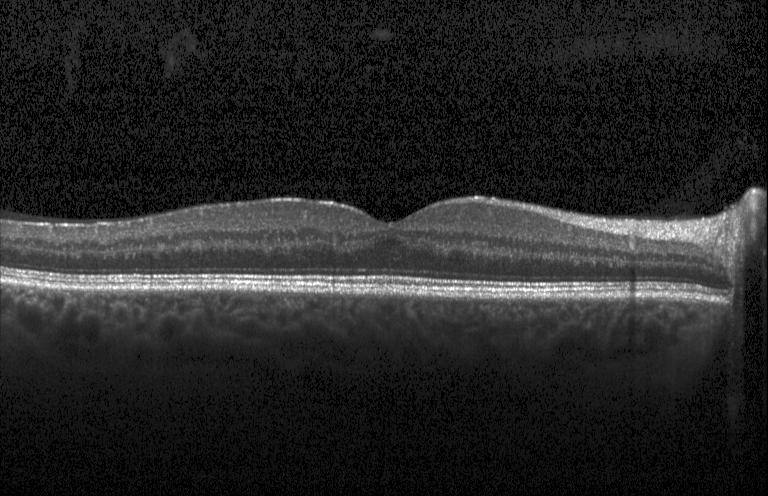 Optical coherence tomography B-scan
Diagnosis: neither CNV, DME, nor drusen.